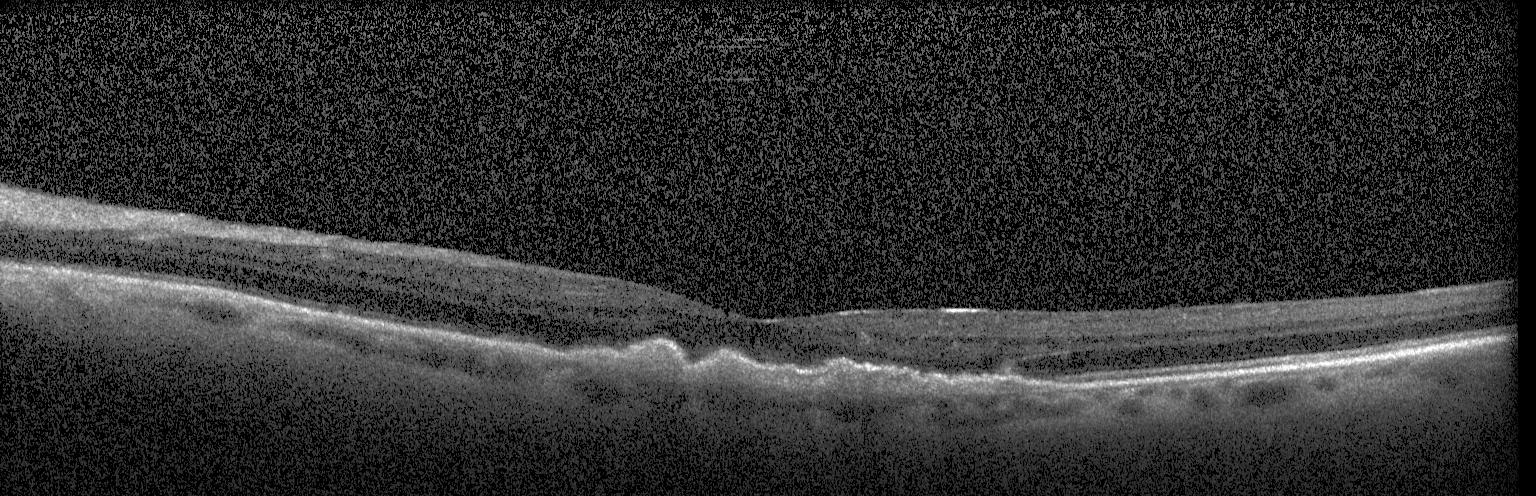

Dx: sub-RPE drusenoid deposits.